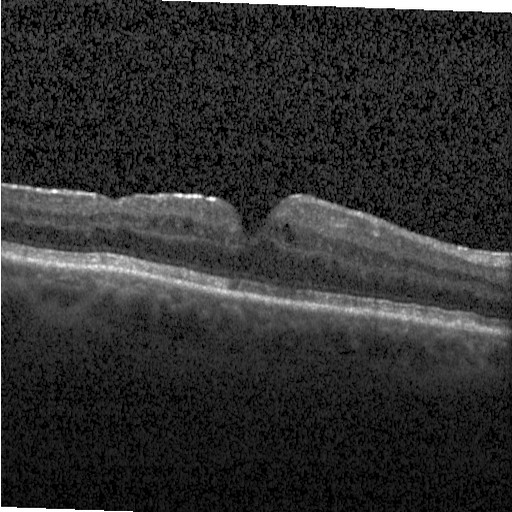 OCT B-scan
Diabetic macular edema.